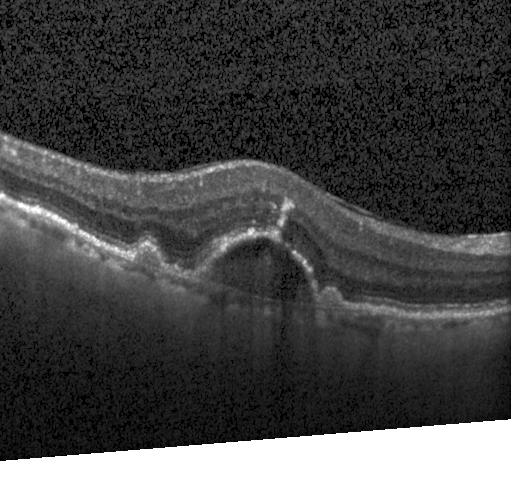 Optical coherence tomography scan
Assessment: choroidal neovascularization (CNV).